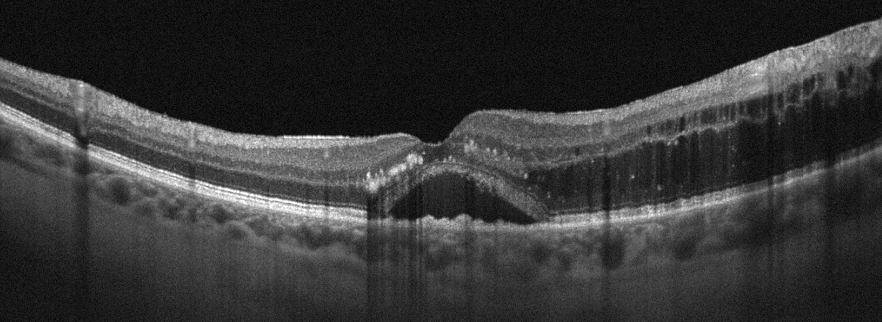
Optical coherence tomography scan.
Retinal vein occlusion (RVO).